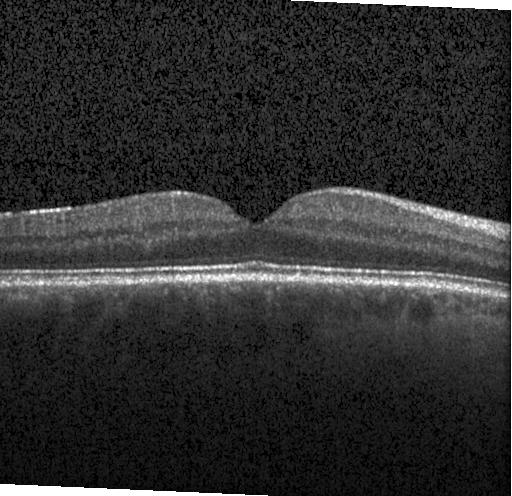
Dx: no CNV, no DME, and no drusen.